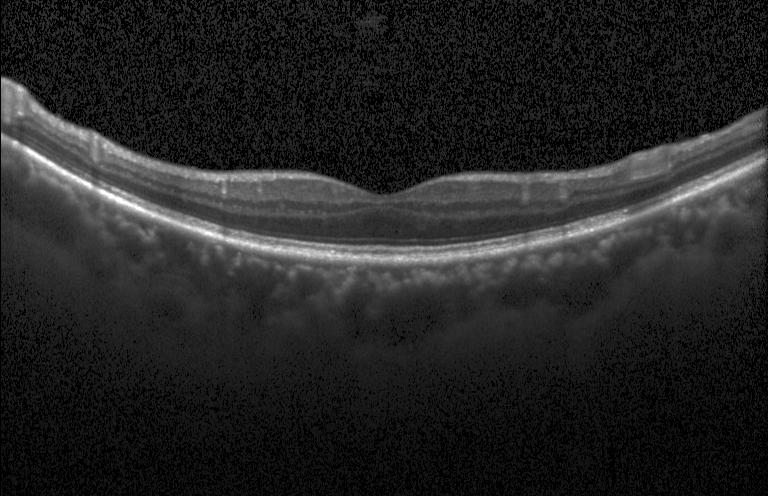 Instrument: Heidelberg Spectralis · OCT line scan. OCT finding: no choroidal neovascularization, no diabetic macular edema, and no drusen.